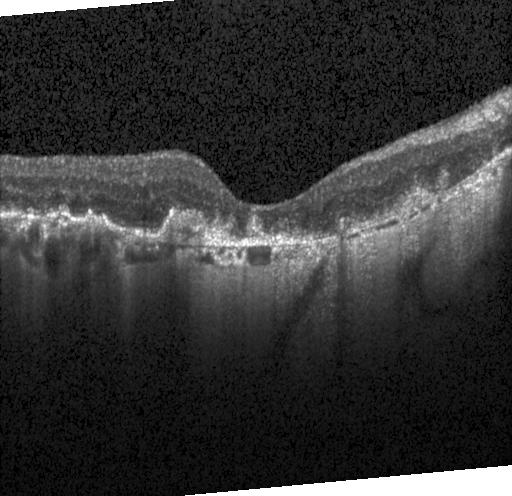
Finding: a choroidal neovascular membrane.